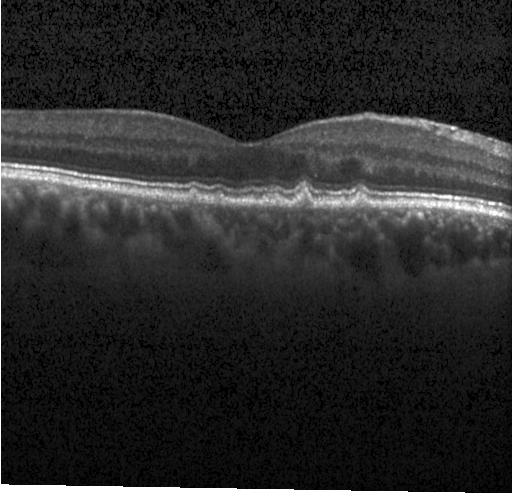
Impression: multiple drusen.